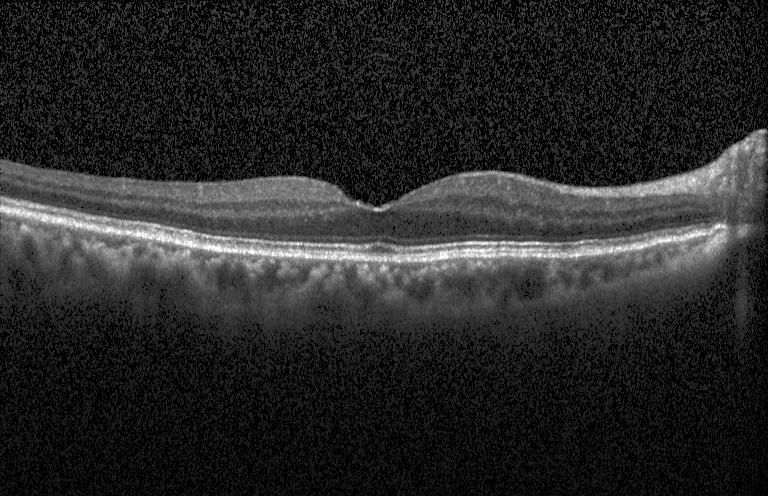

Macular scan. Spectral-domain OCT. OCT line scan
Macular OCT: no CNV, DME, or drusen.